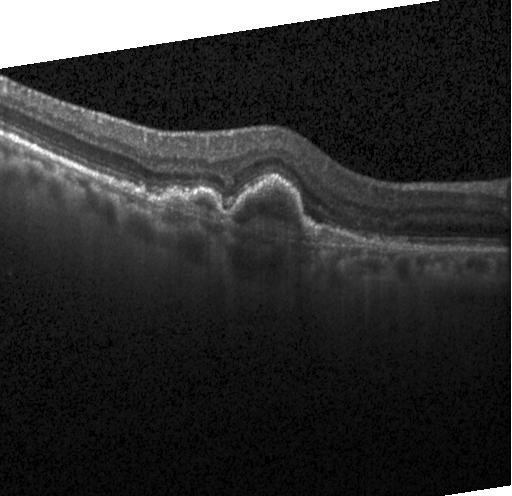

Finding: choroidal neovascularization.